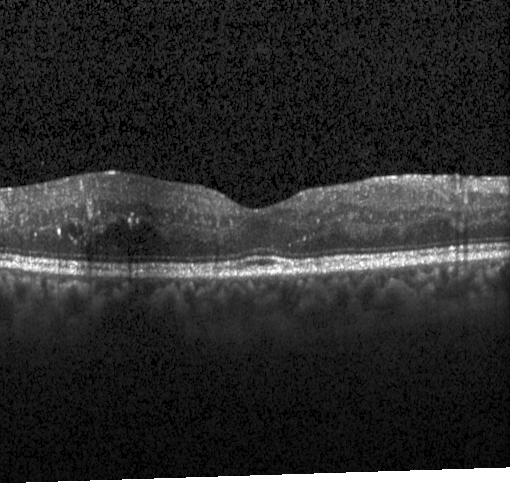

OCT B-scan
Impression: diabetic macular edema.